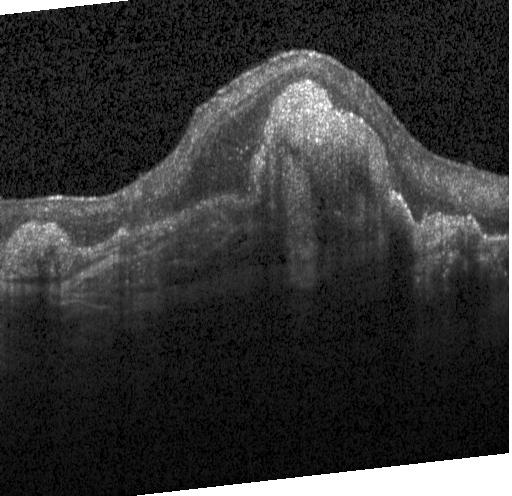

Heidelberg Spectralis. OCT B-scan. SD-OCT.
The scan shows CNV.